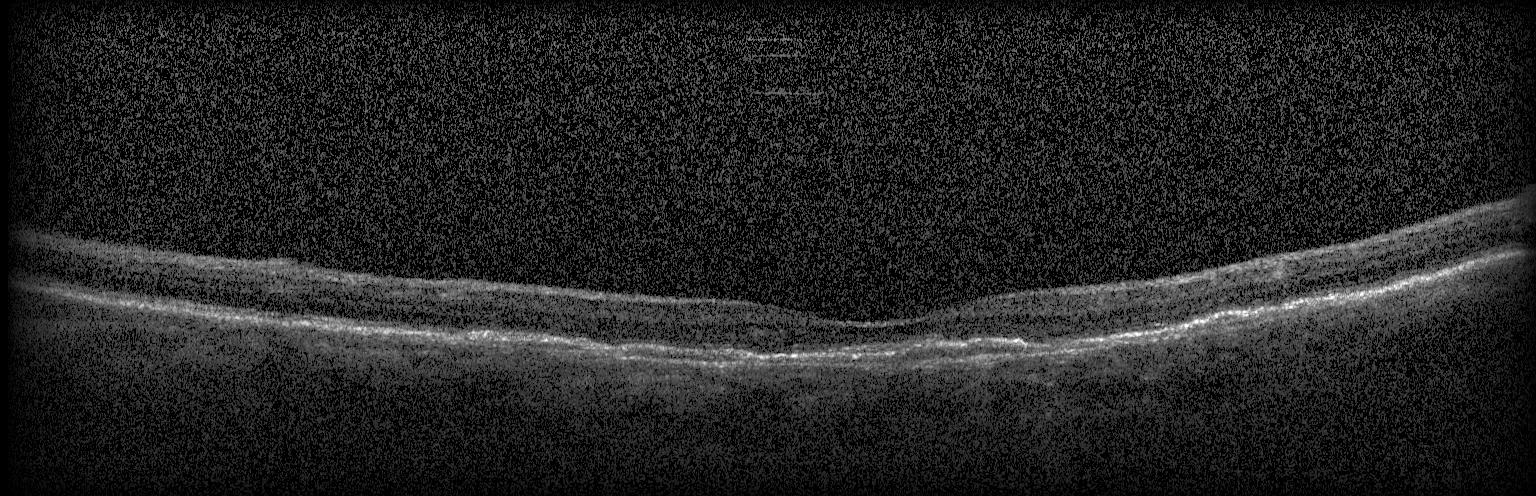 The scan shows choroidal neovascularization.